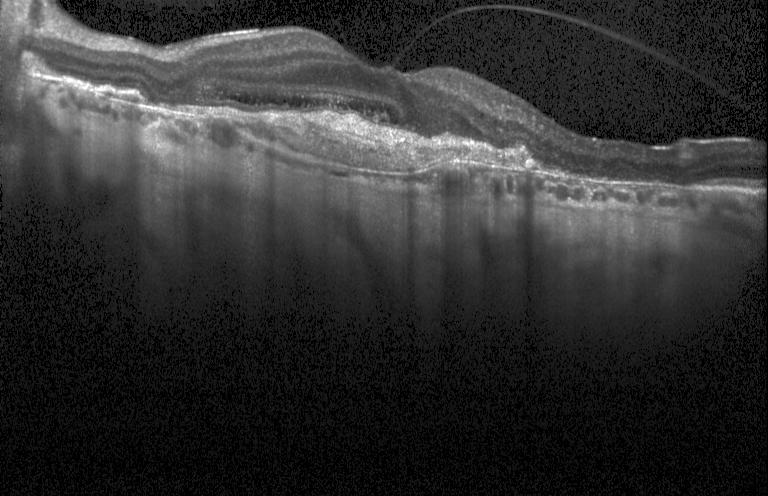

OCT B-scan. CNV.